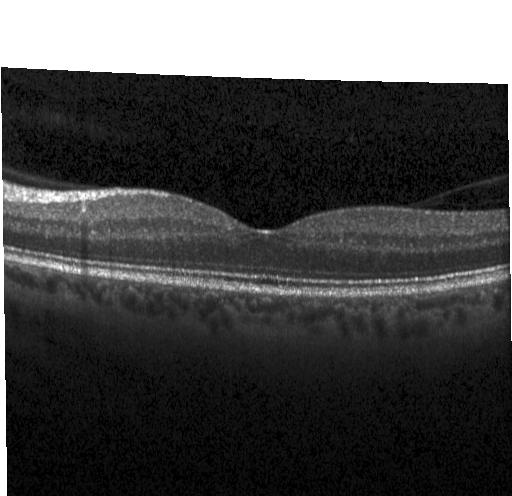
Heidelberg Spectralis, OCT line scan, horizontal scan through the fovea
Assessment: no choroidal neovascularization, diabetic macular edema, or drusen.